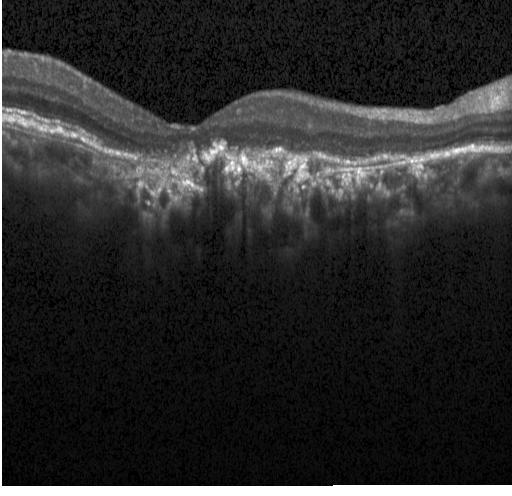
Optical coherence tomography scan · spectral-domain optical coherence tomography
Finding: CNV.